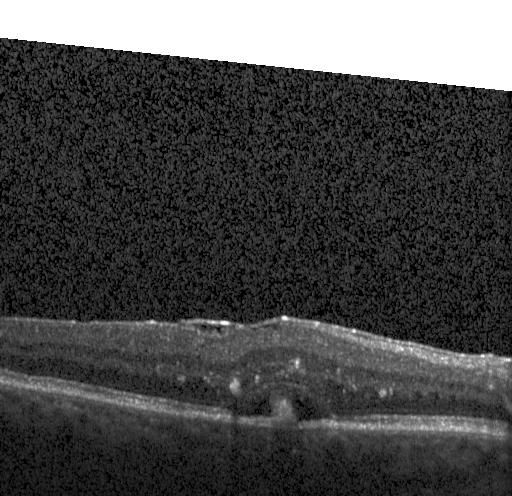 Spectral-domain OCT B-scan: choroidal neovascularization (CNV).